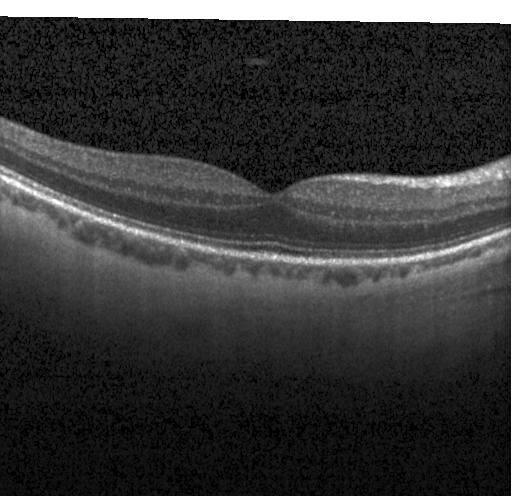

Dx: neither choroidal neovascularization, diabetic macular edema, nor drusen.